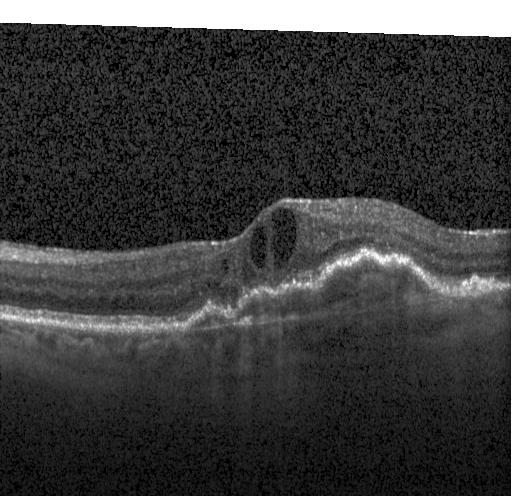

Optical coherence tomography B-scan · Heidelberg Spectralis OCT system. Finding: CNV.